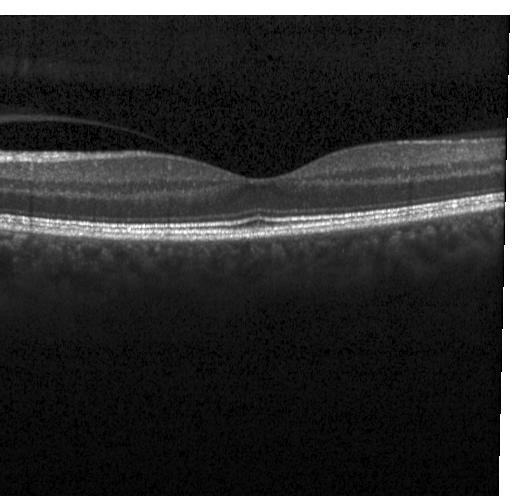

OCT B-scan, SD-OCT.
Impression: no choroidal neovascularization, diabetic macular edema, or drusen.